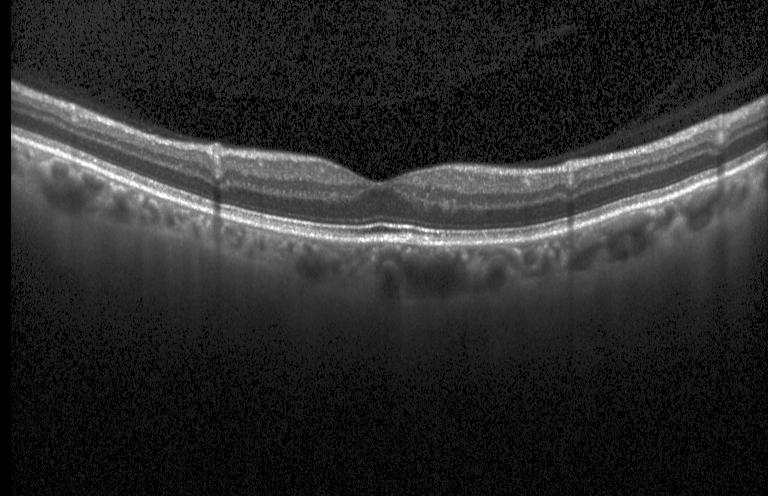 The scan shows sub-RPE drusenoid deposits.